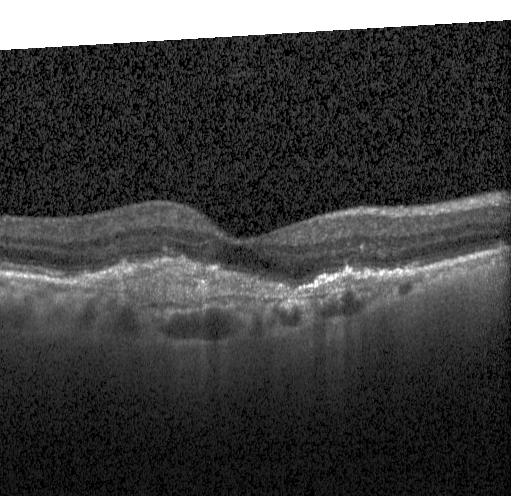 Macular scan. Acquired on a Heidelberg Spectralis. OCT line scan — Assessment: choroidal neovascularization.